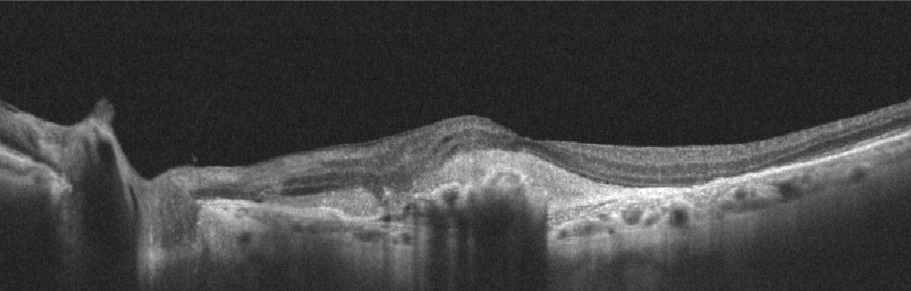
Impression: age-related macular degeneration.